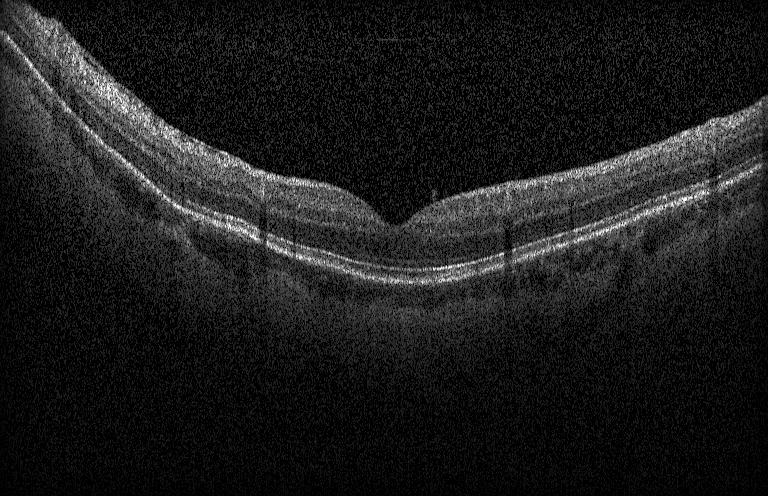

Macular OCT demonstrating no CNV, no DME, and no drusen.